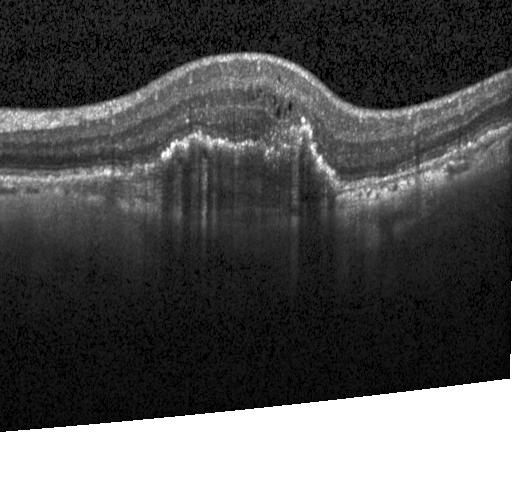

Finding: CNV.